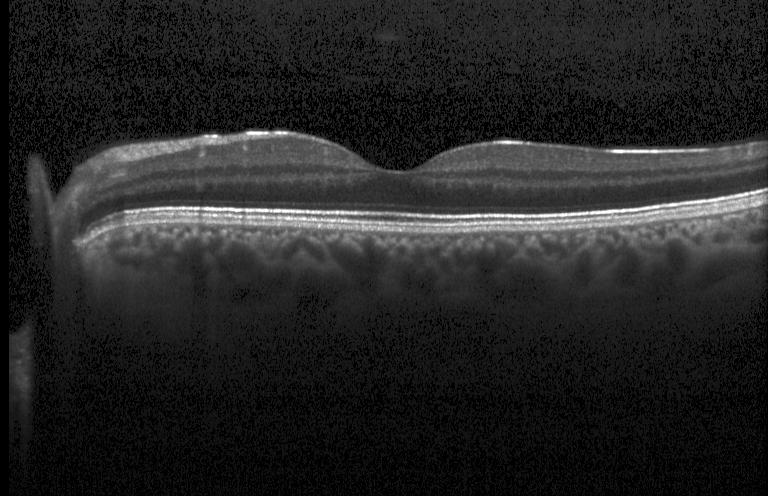
OCT B-scan — The scan shows no CNV, no DME, and no drusen.